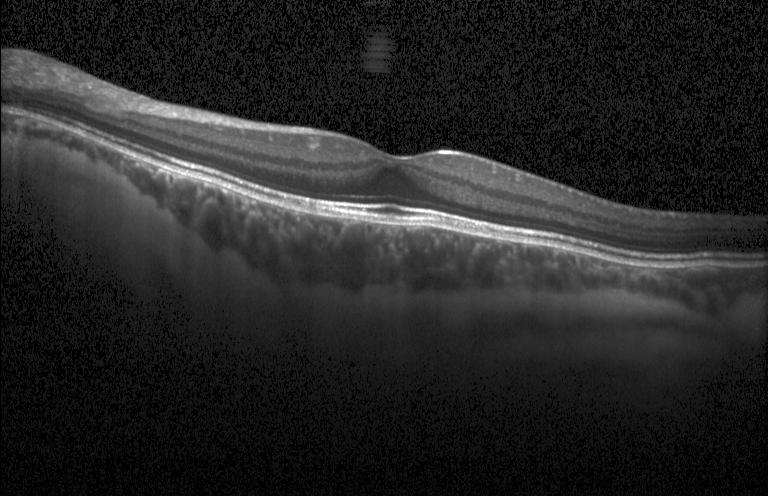

Macular OCT: no CNV, DME, or drusen.